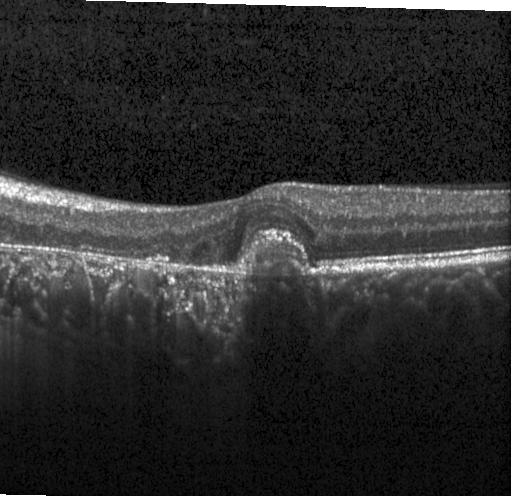

Instrument: Heidelberg Spectralis. Spectral-domain optical coherence tomography. Optical coherence tomography B-scan.
Impression: CNV.